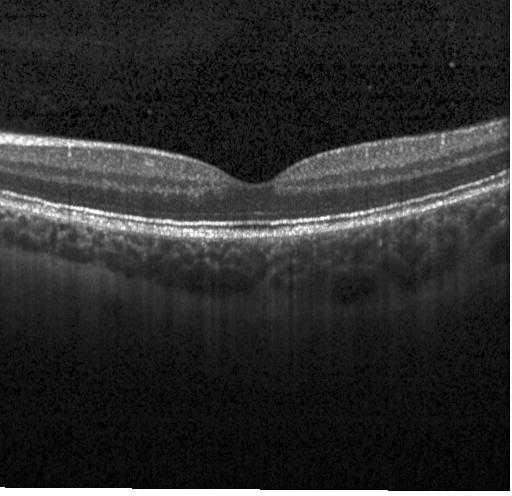

Retinal OCT B-scan · spectral-domain optical coherence tomography
No evidence of choroidal neovascularization, diabetic macular edema, or drusen.